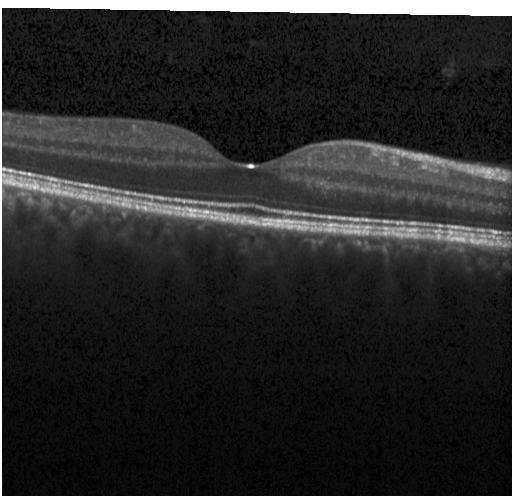 OCT B-scan.
Finding: neither choroidal neovascularization, diabetic macular edema, nor drusen.